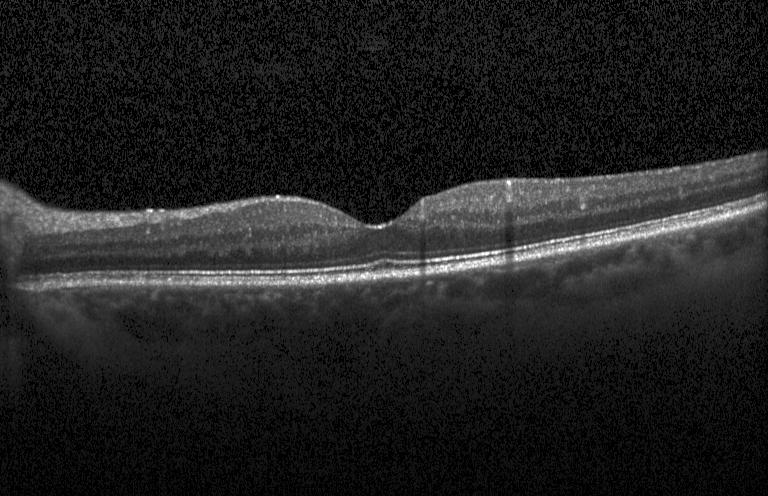

OCT finding: no choroidal neovascularization, diabetic macular edema, or drusen.